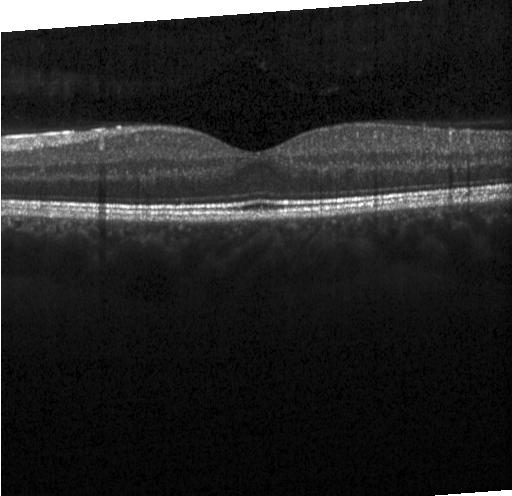 Retinal OCT cross-section, acquired on a Heidelberg Spectralis, horizontal scan through the fovea
OCT finding: neither choroidal neovascularization, diabetic macular edema, nor drusen.